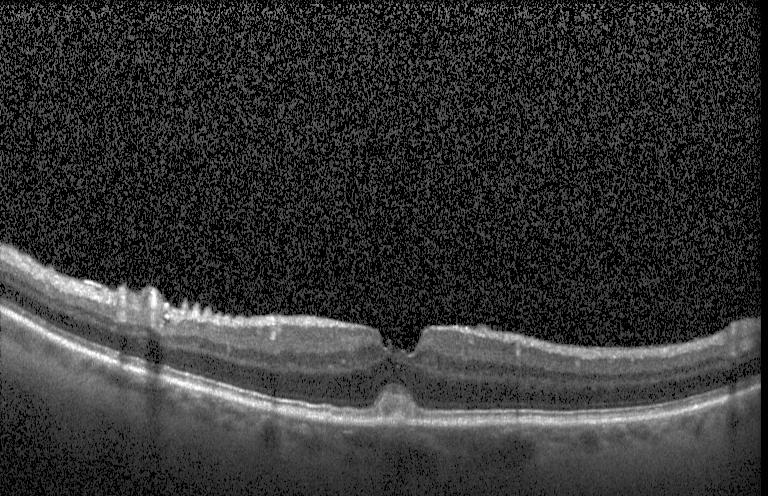
Fovea-centered, optical coherence tomography scan. OCT finding: sub-RPE drusenoid deposits.